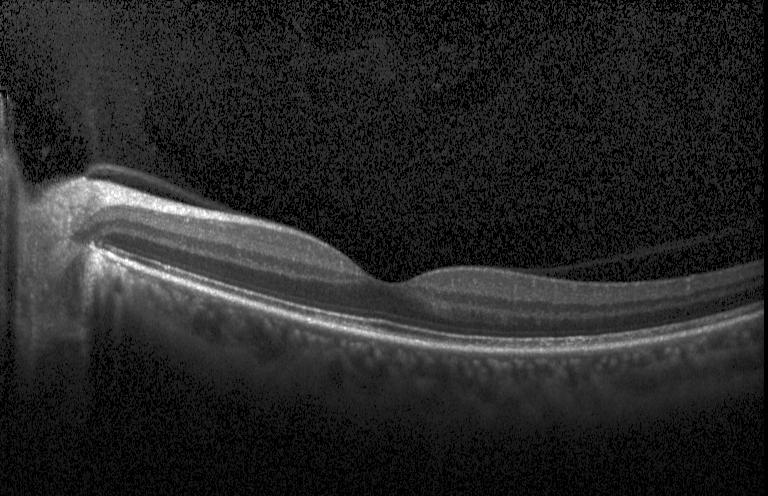 Impression: no evidence of choroidal neovascularization, diabetic macular edema, or drusen.